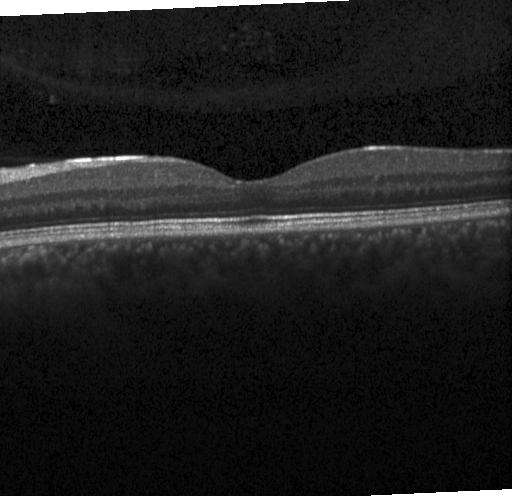
Optical coherence tomography scan.
Impression: no choroidal neovascularization, no diabetic macular edema, and no drusen.